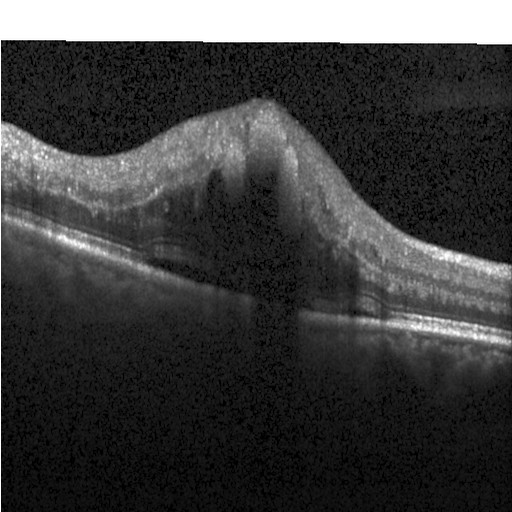

Diagnosis: diabetic macular edema (DME).